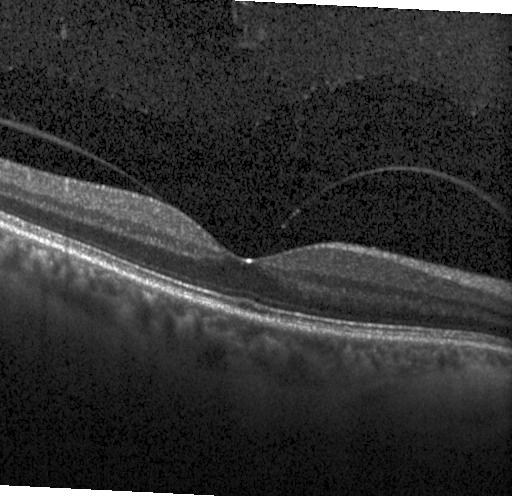

The scan shows neither choroidal neovascularization, diabetic macular edema, nor drusen.